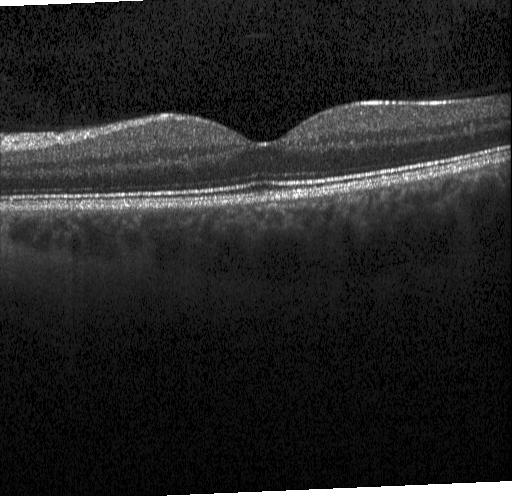 Heidelberg Spectralis OCT system · spectral-domain OCT · optical coherence tomography scan.
Impression: no choroidal neovascularization, diabetic macular edema, or drusen.